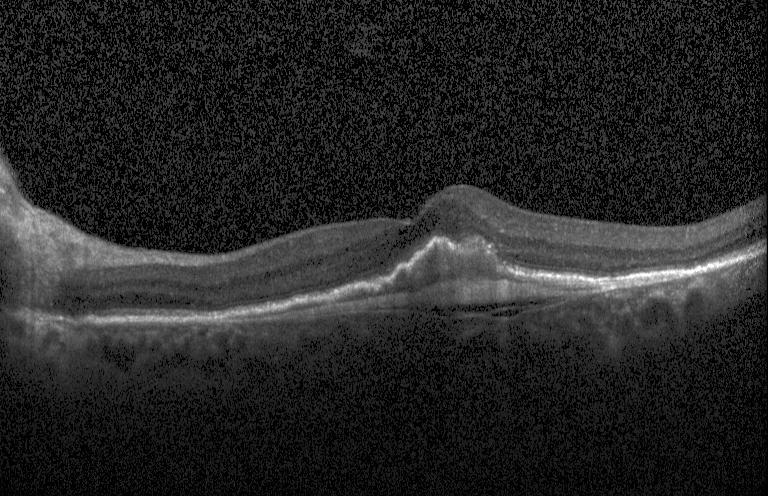 Retinal OCT cross-section, Heidelberg Spectralis. Dx: CNV.